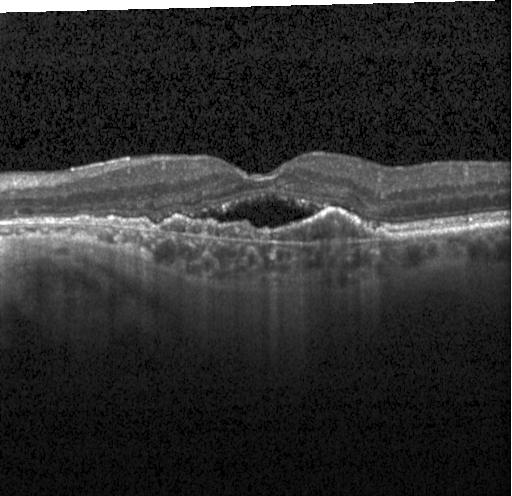

OCT B-scan. Macular scan. SD-OCT — Dx: a choroidal neovascular membrane.